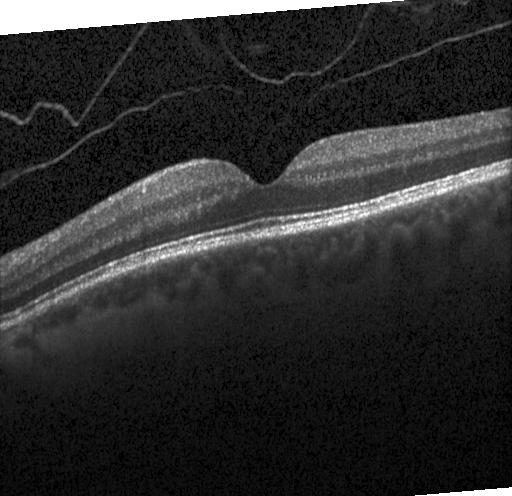
Heidelberg Spectralis · spectral-domain optical coherence tomography · centered on the fovea · OCT line scan. Finding: no evidence of choroidal neovascularization, diabetic macular edema, or drusen.